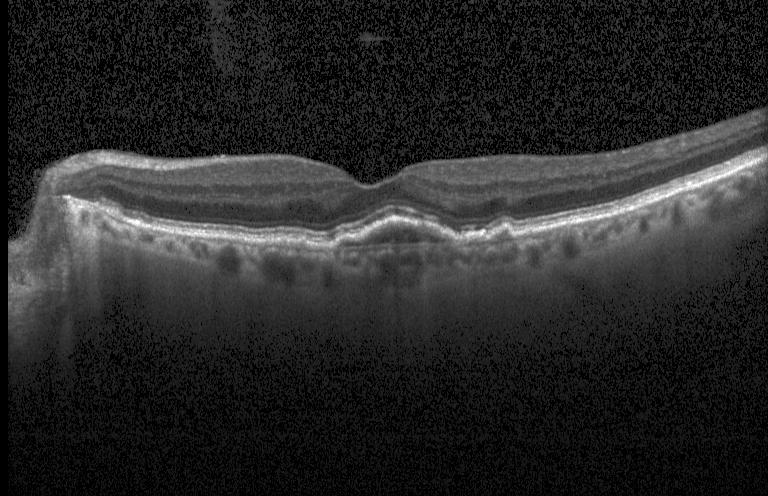
SD-OCT · retinal OCT cross-section. The scan shows CNV.